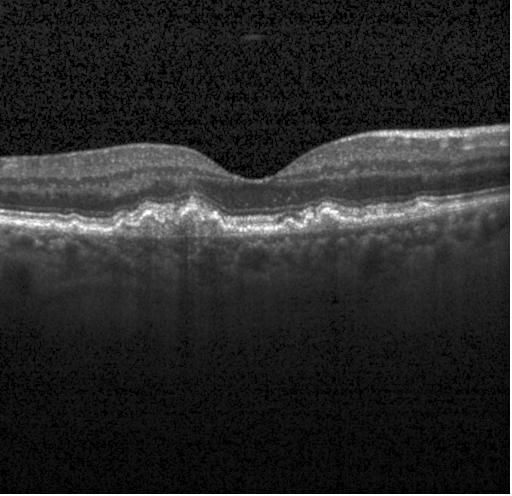 OCT finding: drusen.